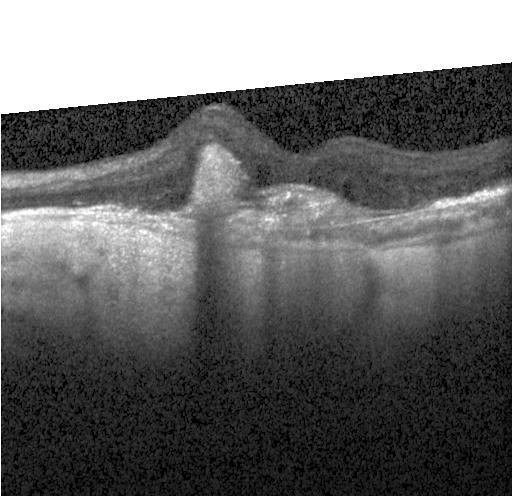 Dx: CNV.